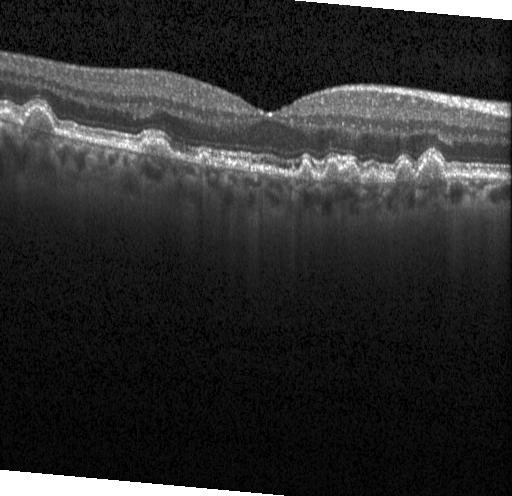 Assessment: drusen.